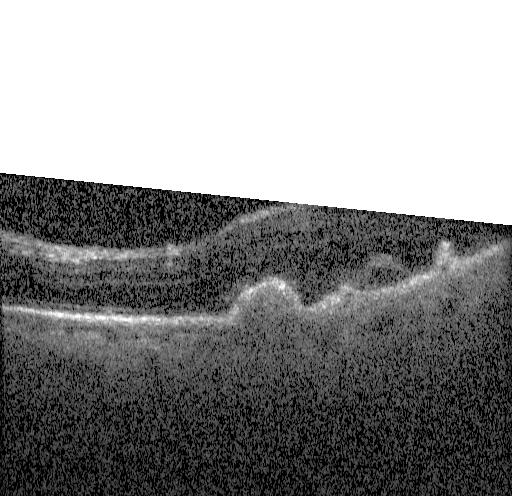
Retinal OCT B-scan
Dx: a choroidal neovascular membrane.